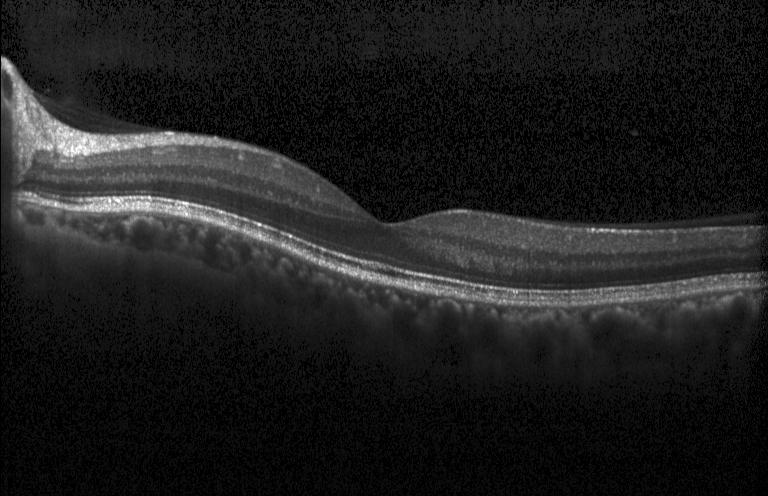
Optical coherence tomography B-scan · instrument: Heidelberg Spectralis. Macular OCT: neither CNV, DME, nor drusen.